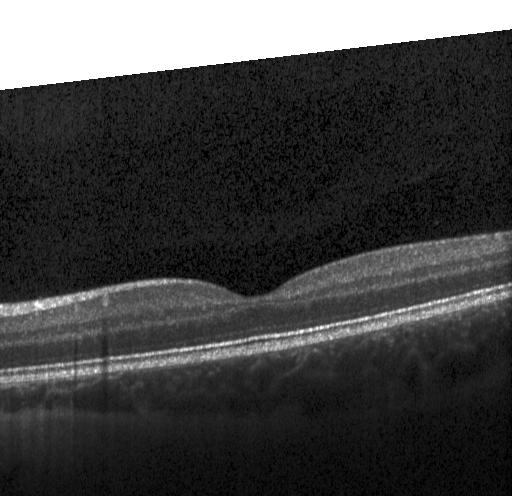

OCT line scan, horizontal scan through the fovea, acquired on a Heidelberg Spectralis. Assessment: no choroidal neovascularization, no diabetic macular edema, and no drusen.